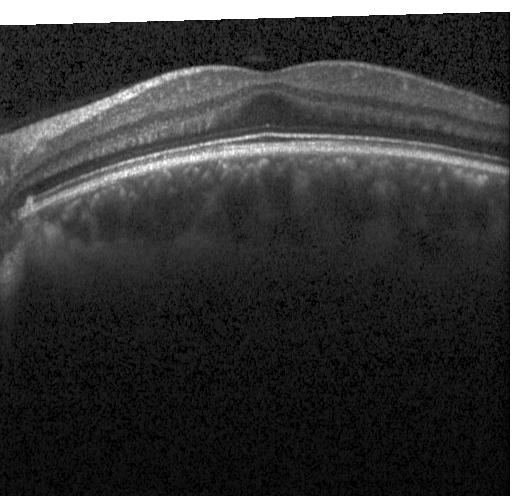

Retinal OCT cross-section — OCT finding: no evidence of CNV, DME, or drusen.